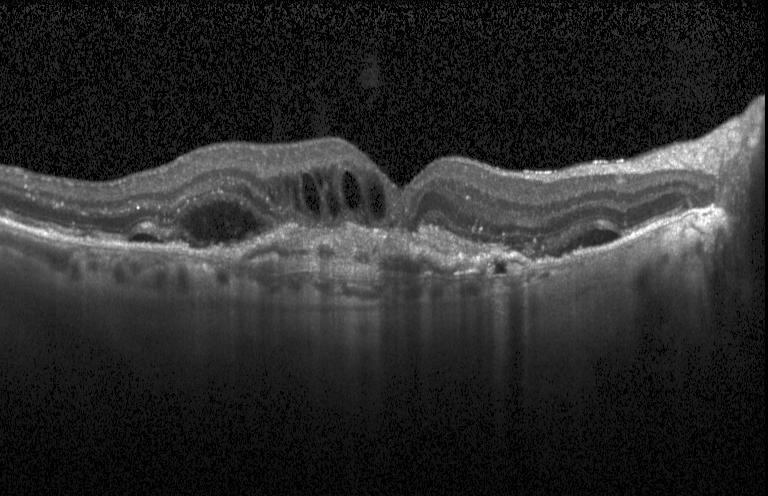 Macular OCT demonstrating a choroidal neovascular membrane.